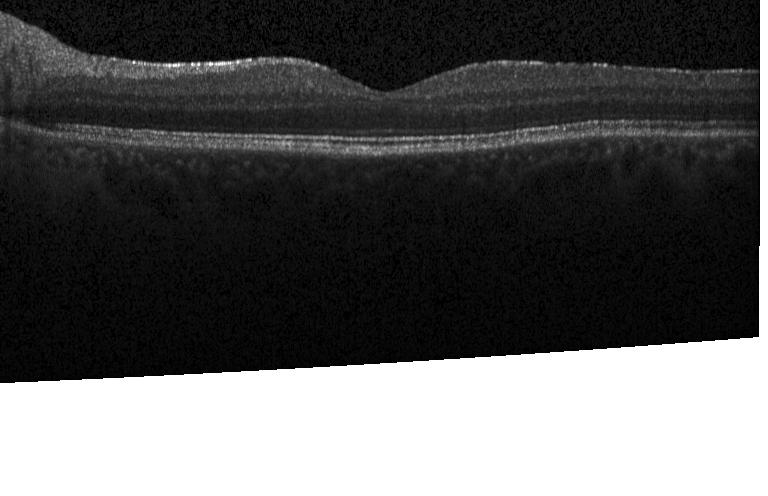 Fovea-centered · spectral-domain OCT · OCT B-scan · instrument: Heidelberg Spectralis.
Impression: no evidence of choroidal neovascularization, diabetic macular edema, or drusen.